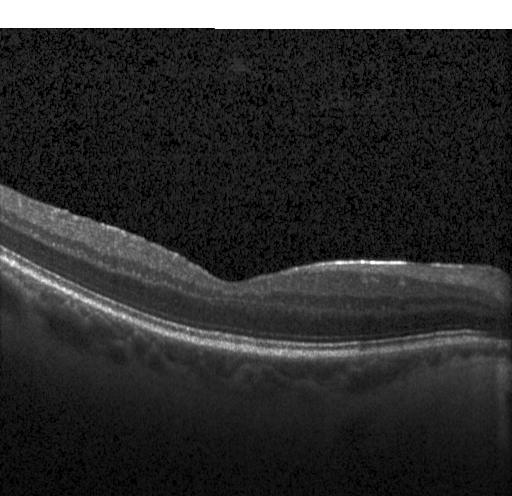

OCT line scan.
No evidence of CNV, DME, or drusen.